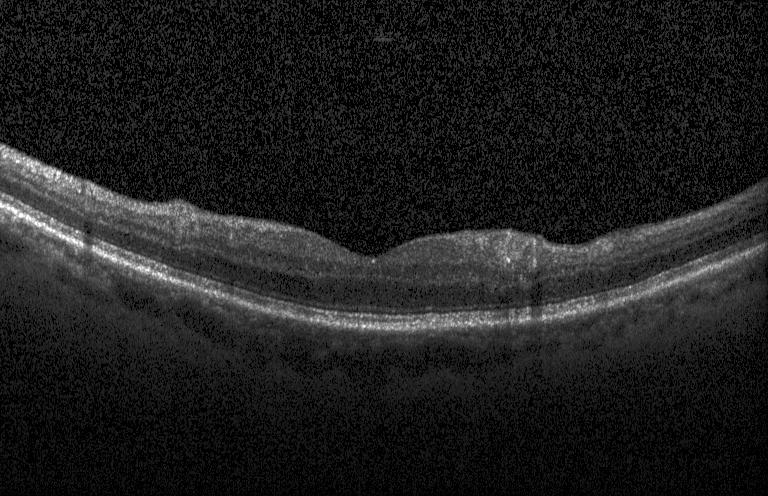

Through the macula; OCT line scan; spectral-domain optical coherence tomography; instrument: Heidelberg Spectralis. Impression: neither CNV, DME, nor drusen.